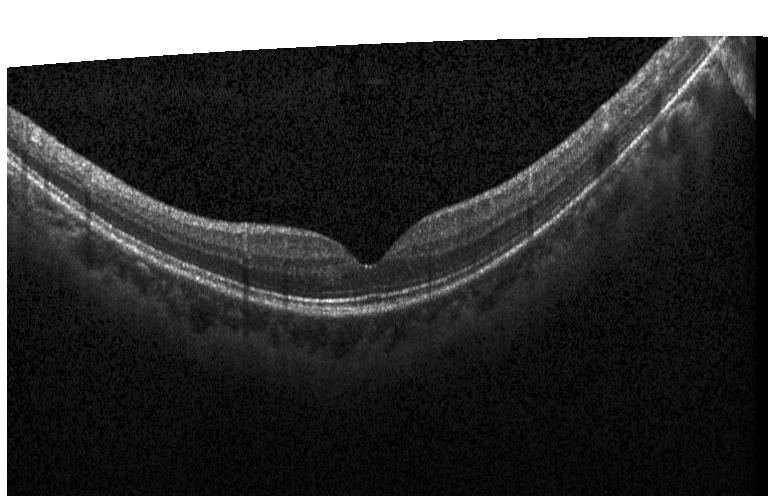

Optical coherence tomography B-scan
Diagnosis: no evidence of choroidal neovascularization, diabetic macular edema, or drusen.